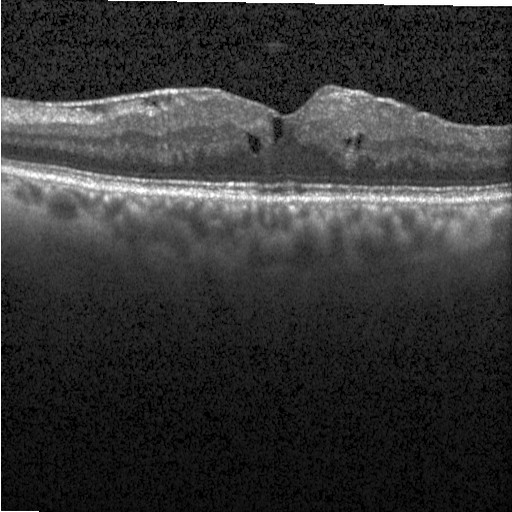 Fovea-centered · Heidelberg Spectralis OCT system · OCT line scan · spectral-domain OCT. Impression: diabetic macular edema.